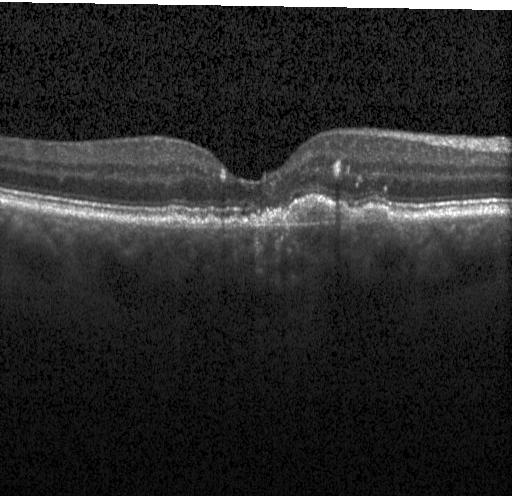

Assessment: choroidal neovascularization (CNV).